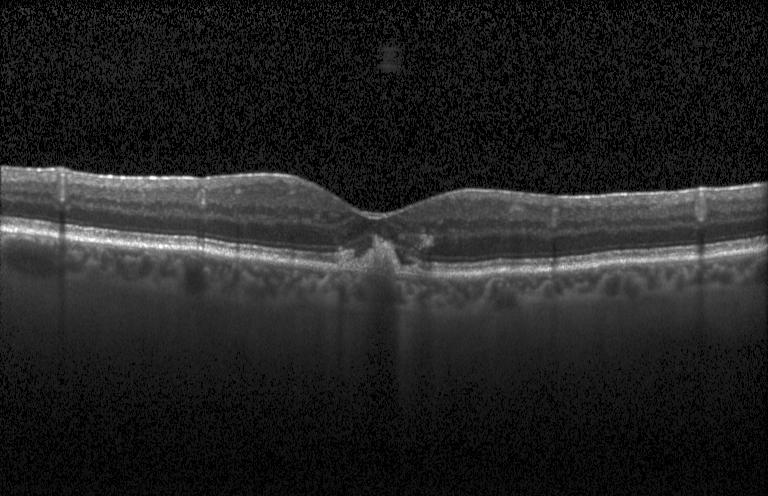
Instrument: Heidelberg Spectralis · OCT B-scan
Finding: choroidal neovascularization (CNV).